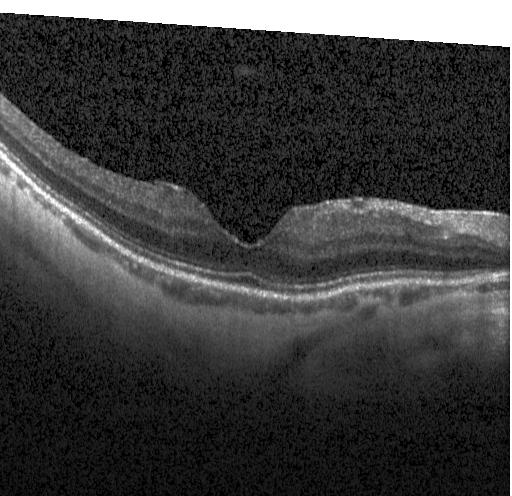

OCT line scan; instrument: Heidelberg Spectralis.
Macular OCT: no evidence of CNV, DME, or drusen.